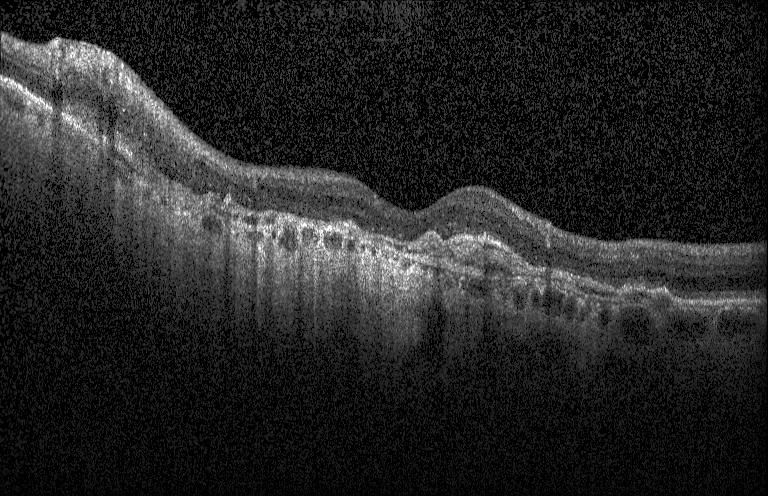
OCT B-scan. SD-OCT. Diagnosis: a choroidal neovascular membrane.